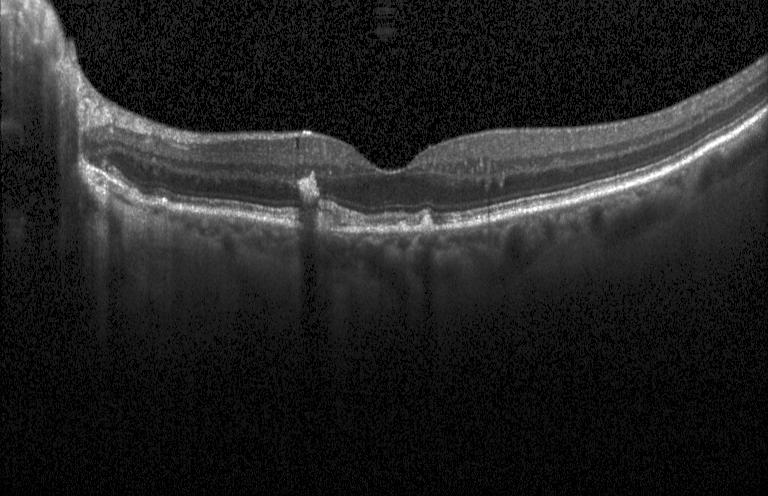

Optical coherence tomography B-scan · spectral-domain OCT · through the macula. Finding: drusen.